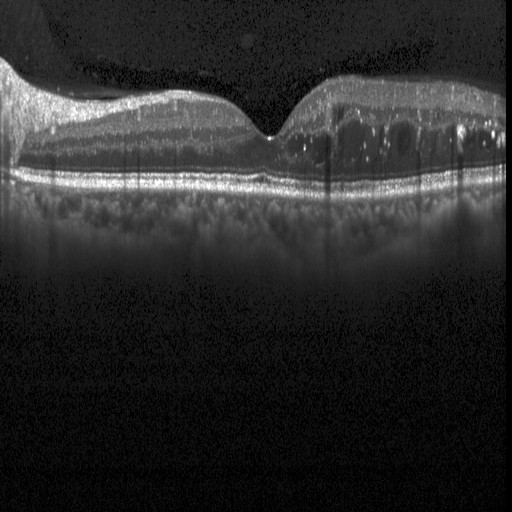

Retinal OCT B-scan · SD-OCT.
Finding: diabetic macular edema.